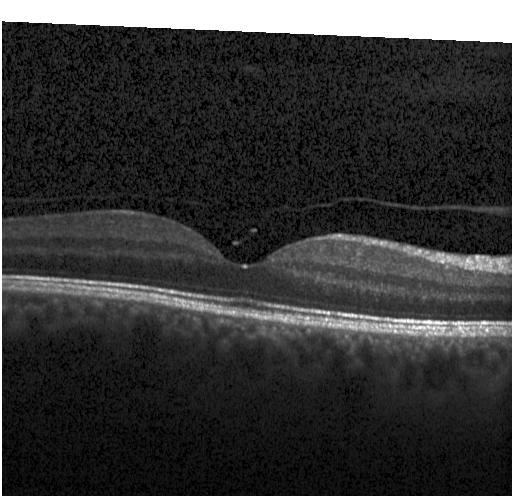 Impression: neither CNV, DME, nor drusen.